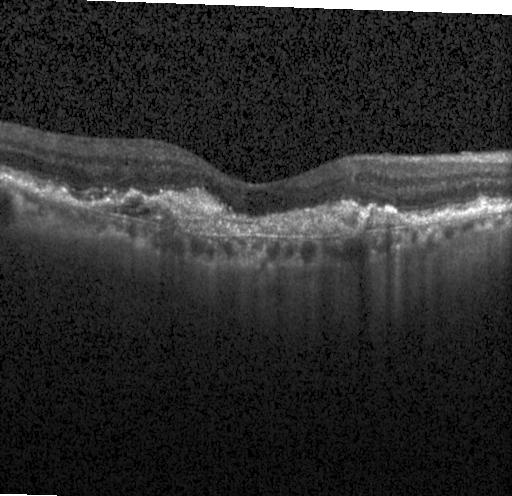 Instrument: Heidelberg Spectralis · through the macula · spectral-domain OCT · OCT B-scan — Macular OCT: CNV.